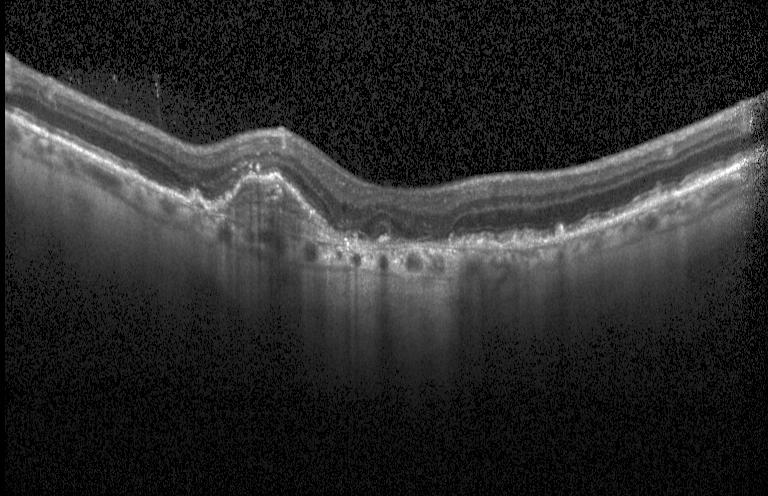

Spectral-domain OCT · optical coherence tomography B-scan · Heidelberg Spectralis · macular scan. Impression: choroidal neovascularization (CNV).